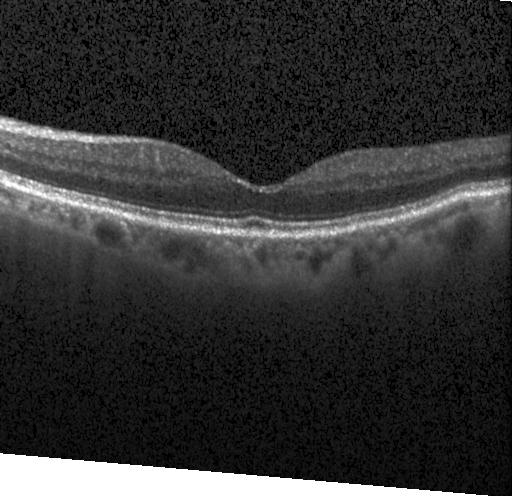 Heidelberg Spectralis OCT system · centered on the fovea · spectral-domain optical coherence tomography · retinal OCT B-scan
Finding: no evidence of CNV, DME, or drusen.